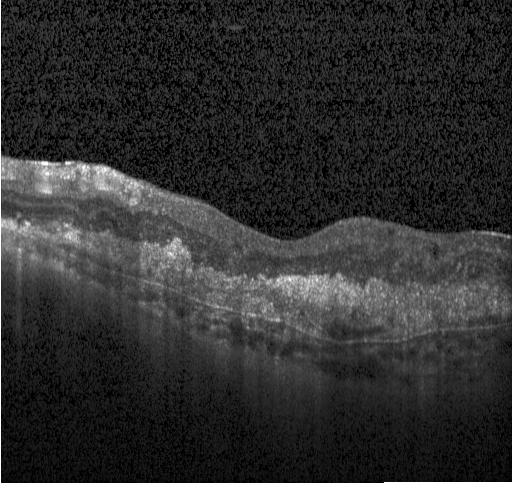
OCT line scan; acquired on a Heidelberg Spectralis; SD-OCT — Assessment: CNV.